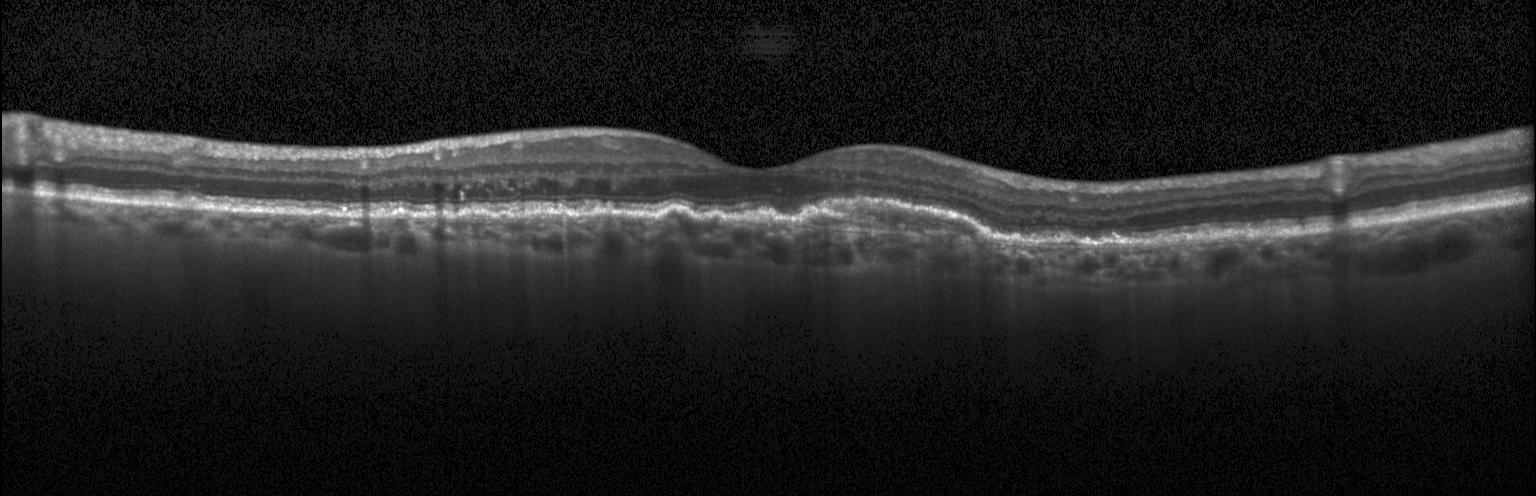

The scan shows a choroidal neovascular membrane.